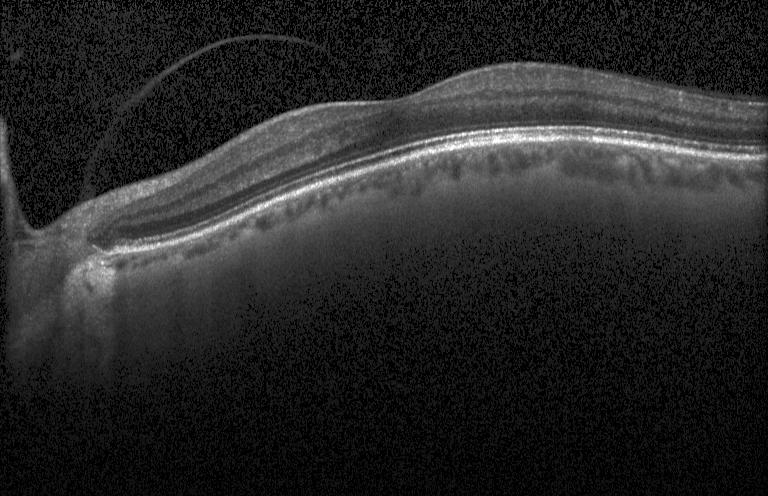 Optical coherence tomography B-scan. SD-OCT. Through the macula. Heidelberg Spectralis.
Finding: no choroidal neovascularization, no diabetic macular edema, and no drusen.